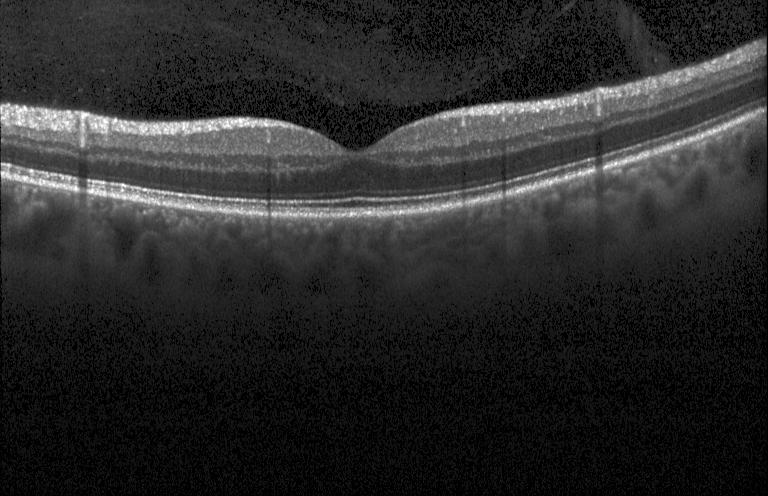

Finding: neither choroidal neovascularization, diabetic macular edema, nor drusen.